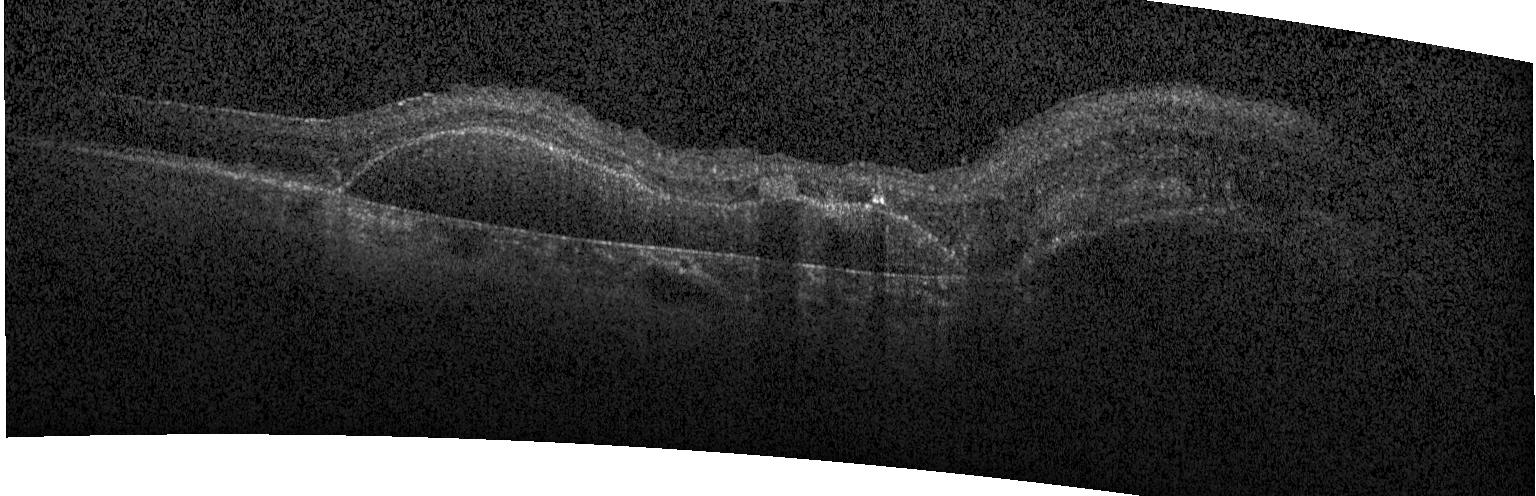
Optical coherence tomography B-scan · SD-OCT — The scan shows a choroidal neovascular membrane.